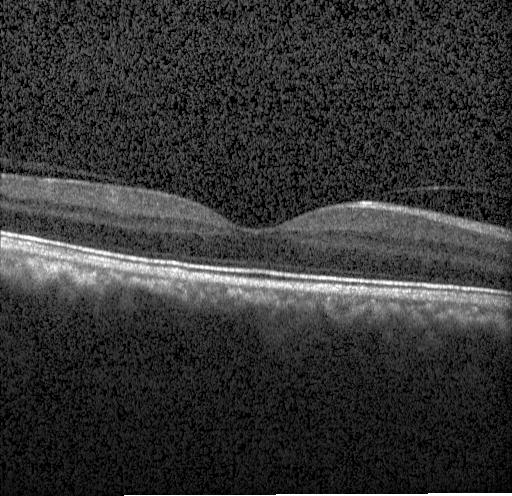 Optical coherence tomography scan; acquired on a Heidelberg Spectralis
OCT finding: no choroidal neovascularization, diabetic macular edema, or drusen.